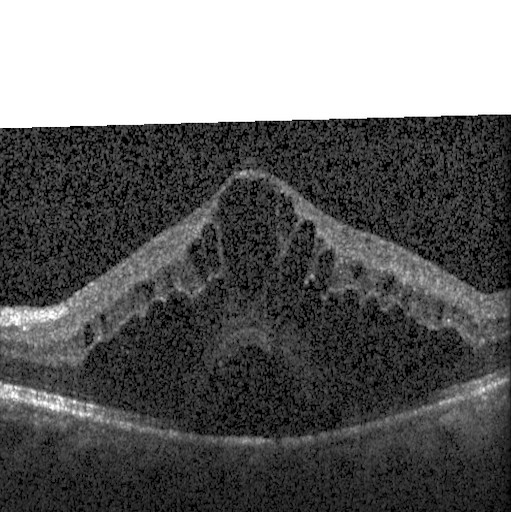 Dx: DME.